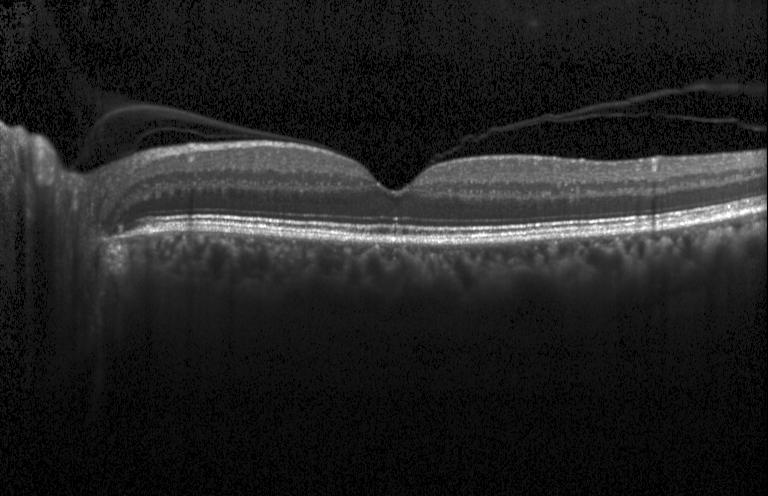
Macular OCT: no evidence of choroidal neovascularization, diabetic macular edema, or drusen.